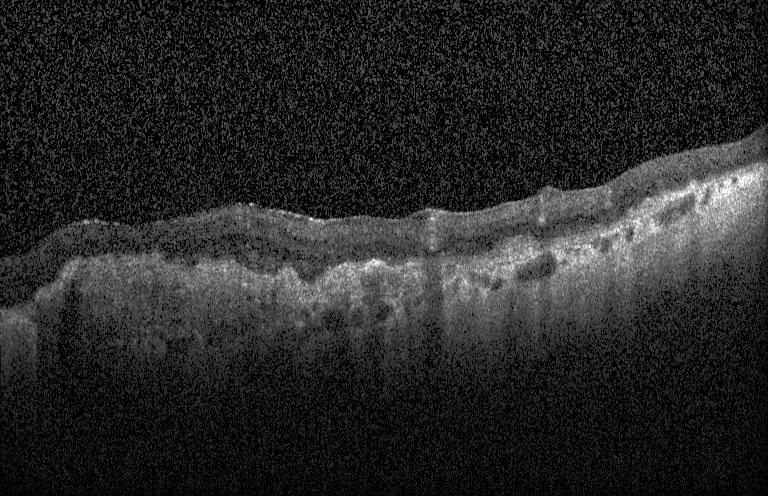
Spectral-domain OCT · Heidelberg Spectralis OCT system · fovea-centered · retinal OCT B-scan
OCT finding: choroidal neovascularization.